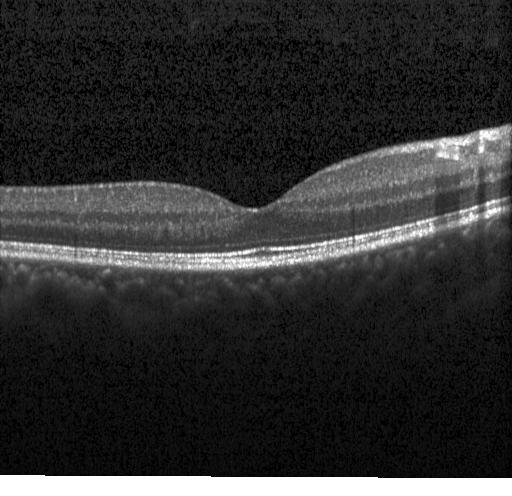
Spectral-domain optical coherence tomography. Acquired on a Heidelberg Spectralis. Retinal OCT cross-section. Through the macula.
The scan shows neither CNV, DME, nor drusen.